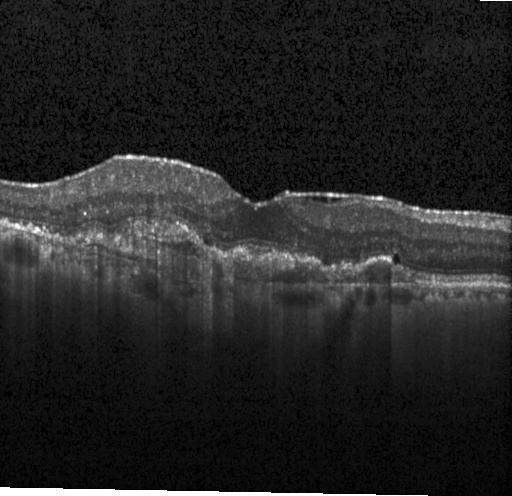
Optical coherence tomography scan; Heidelberg Spectralis OCT system; centered on the fovea; spectral-domain optical coherence tomography.
The scan shows choroidal neovascularization (CNV).